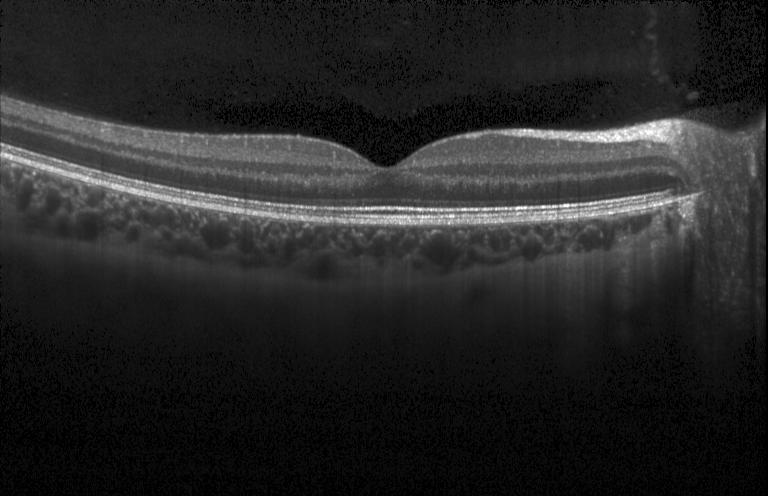 OCT B-scan — This B-scan demonstrates neither choroidal neovascularization, diabetic macular edema, nor drusen.